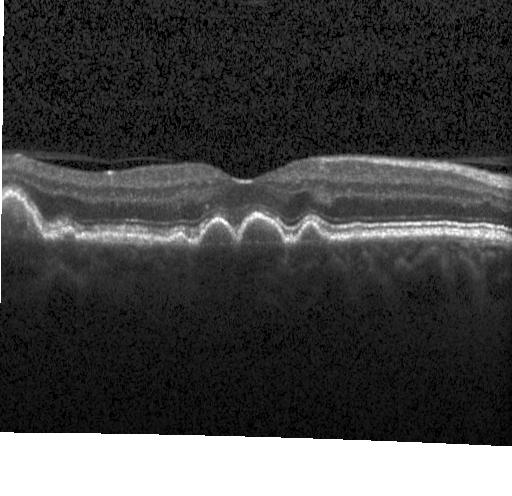
Centered on the fovea. Acquired on a Heidelberg Spectralis. SD-OCT. OCT B-scan.
Diagnosis: multiple drusen.